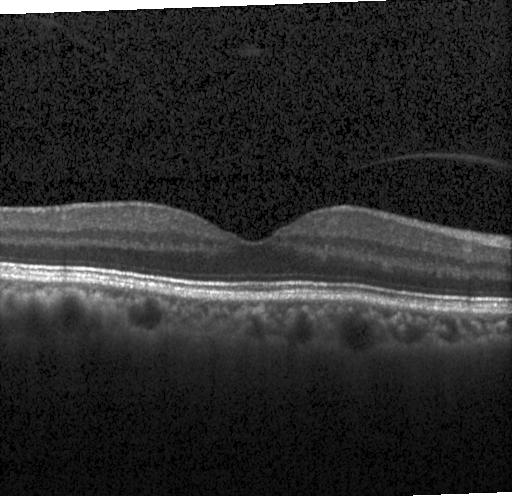 Retinal OCT cross-section
Impression: neither CNV, DME, nor drusen.